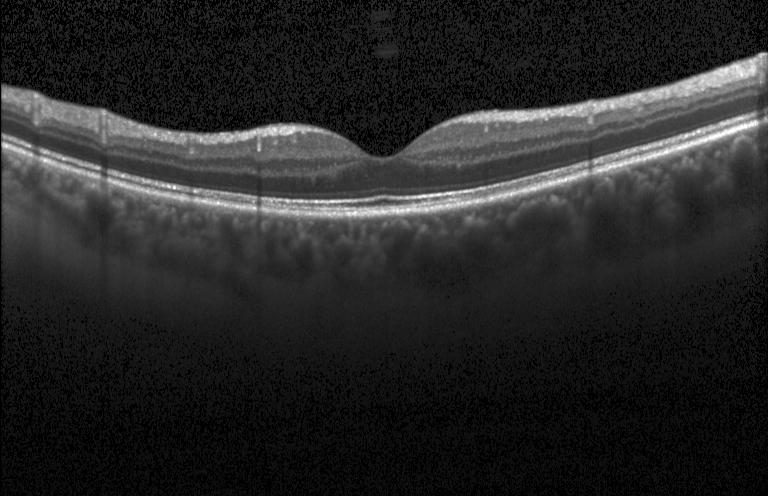 Optical coherence tomography scan · Heidelberg Spectralis OCT system · SD-OCT · through the macula. Finding: no evidence of choroidal neovascularization, diabetic macular edema, or drusen.